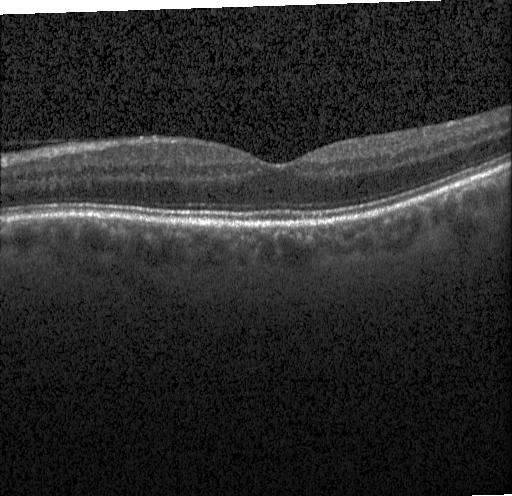 Retinal OCT cross-section; macular scan; acquired on a Heidelberg Spectralis; spectral-domain optical coherence tomography. The scan shows no choroidal neovascularization, no diabetic macular edema, and no drusen.